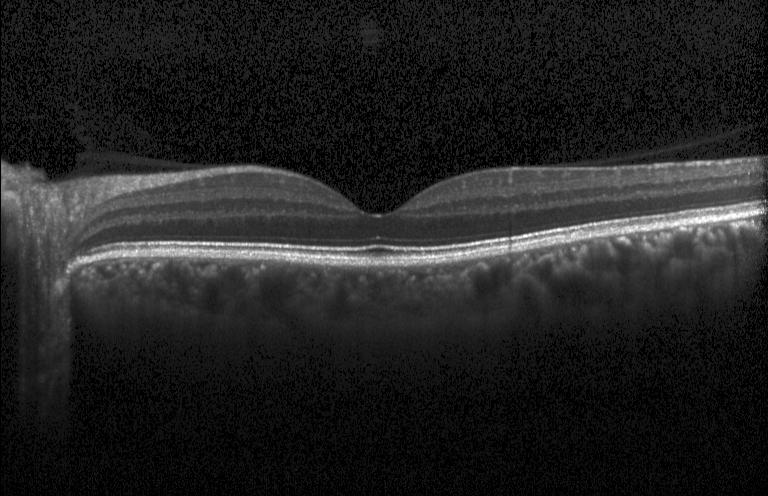
Impression: neither choroidal neovascularization, diabetic macular edema, nor drusen.